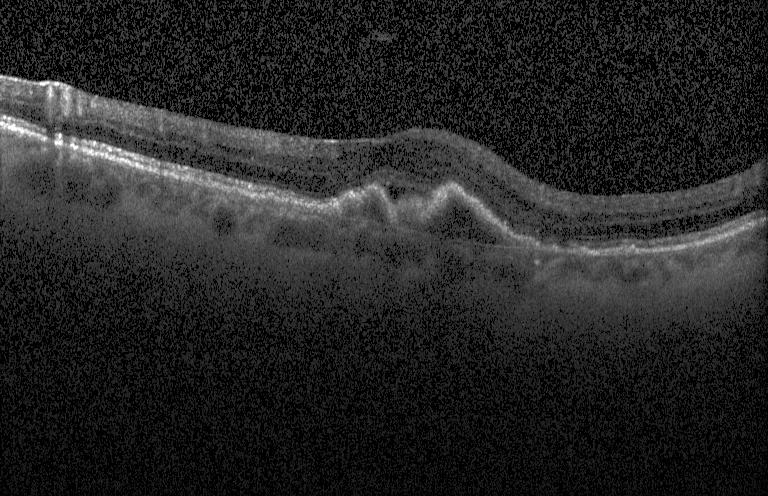 Heidelberg Spectralis OCT system; OCT line scan; macular scan; spectral-domain optical coherence tomography
Impression: a choroidal neovascular membrane.